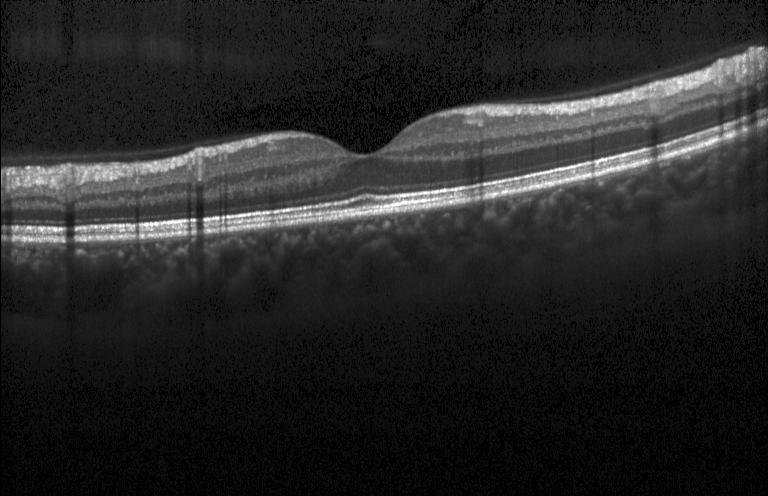 Diagnosis: no evidence of choroidal neovascularization, diabetic macular edema, or drusen.